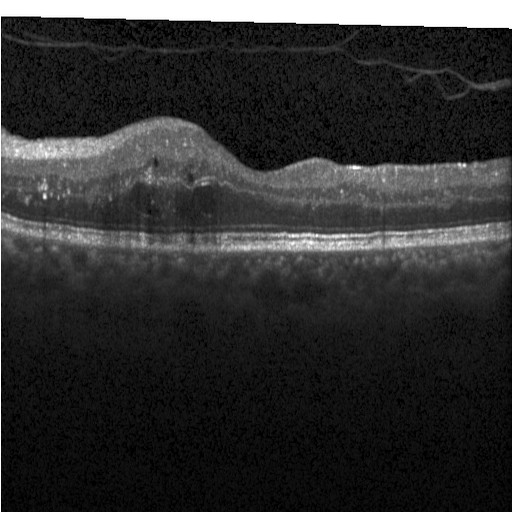 Macular OCT demonstrating diabetic macular edema.